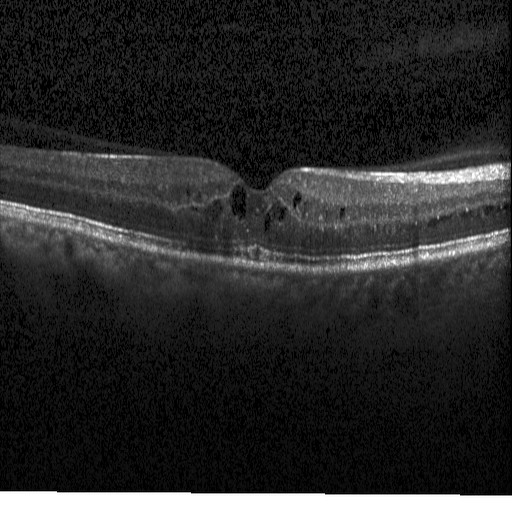
Acquired on a Heidelberg Spectralis · spectral-domain optical coherence tomography · fovea-centered · OCT B-scan
The scan shows DME.